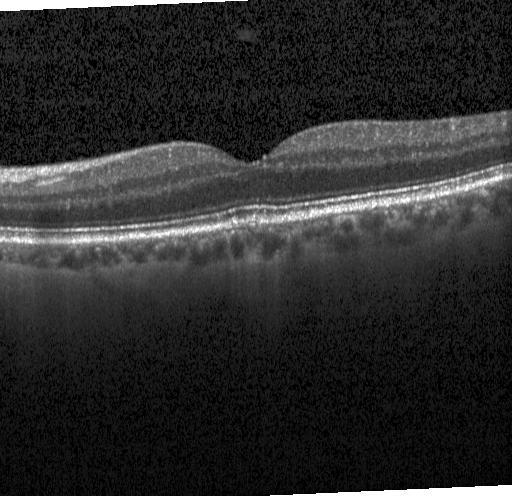

OCT B-scan showing no evidence of choroidal neovascularization, diabetic macular edema, or drusen.